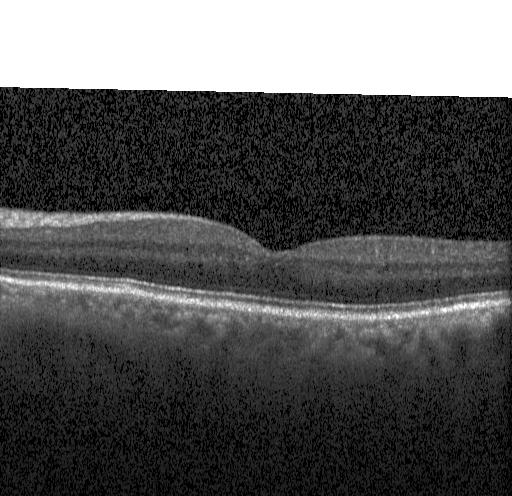 Diagnosis: no CNV, no DME, and no drusen.